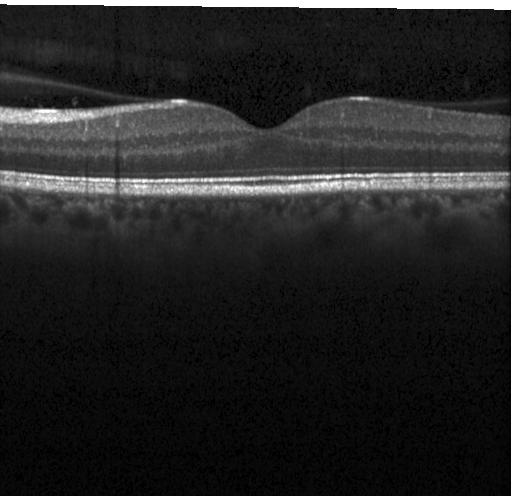

Finding: no CNV, no DME, and no drusen.